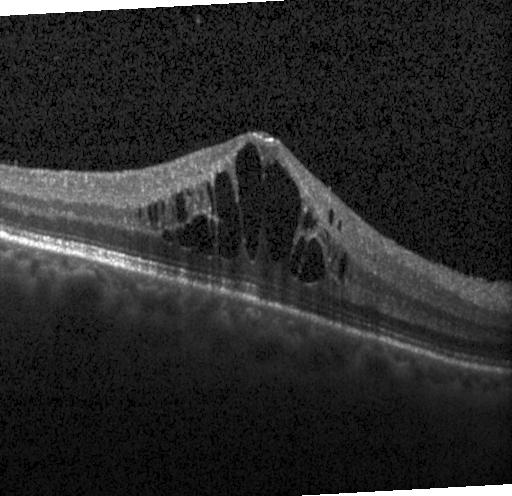

Acquired on a Heidelberg Spectralis. Spectral-domain OCT. OCT B-scan. Horizontal scan through the fovea. Diagnosis: DME.